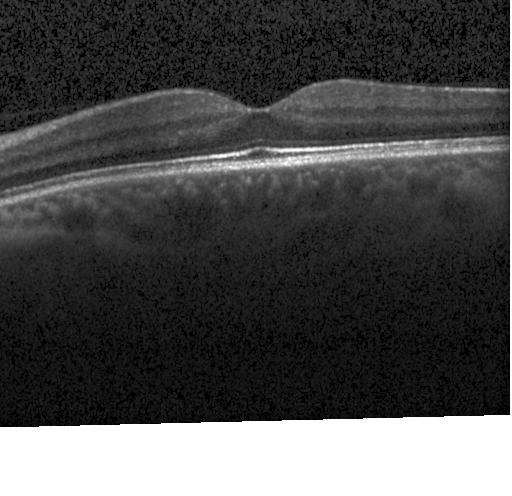
Heidelberg Spectralis OCT system; retinal OCT B-scan; fovea-centered
Assessment: no evidence of CNV, DME, or drusen.